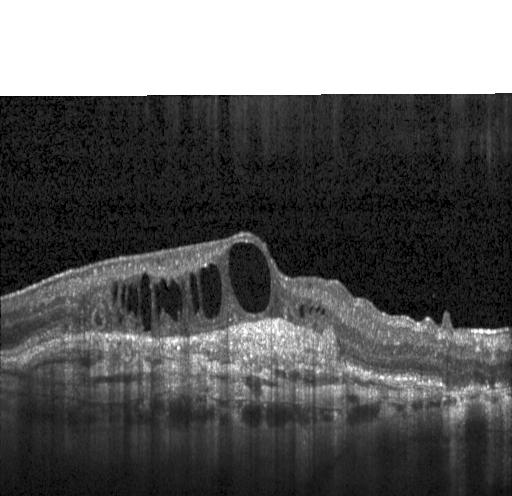 Acquired on a Heidelberg Spectralis · retinal OCT cross-section · horizontal scan through the fovea · spectral-domain OCT — Diagnosis: a choroidal neovascular membrane.